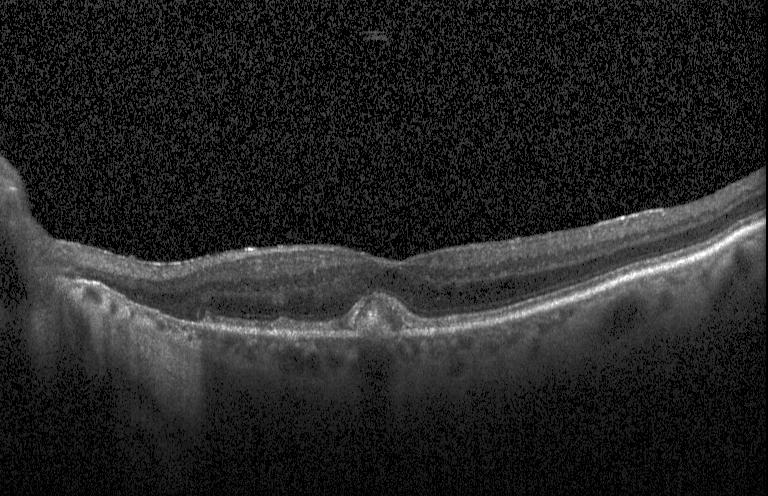 Macular OCT: CNV.